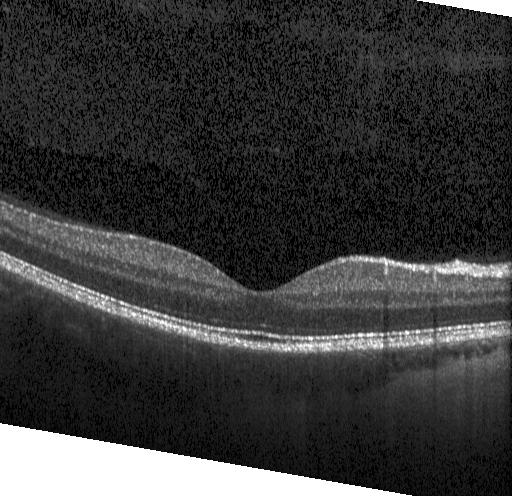
SD-OCT. Heidelberg Spectralis OCT system. Horizontal scan through the fovea. Retinal OCT B-scan — Neither choroidal neovascularization, diabetic macular edema, nor drusen.